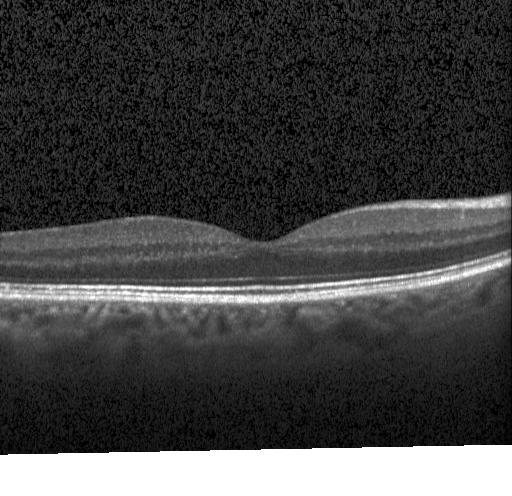
Impression: no choroidal neovascularization, diabetic macular edema, or drusen.